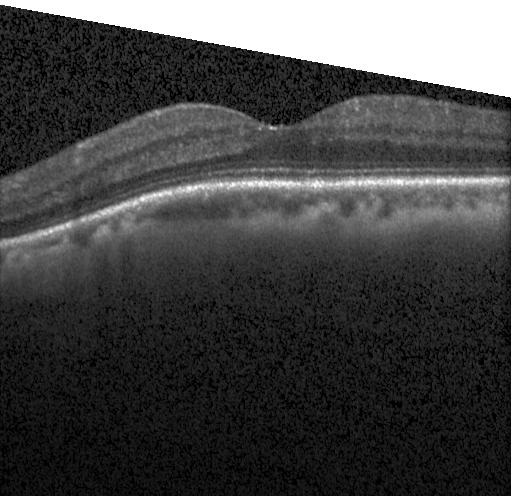
SD-OCT · OCT line scan · Heidelberg Spectralis OCT system
Finding: no choroidal neovascularization, no diabetic macular edema, and no drusen.